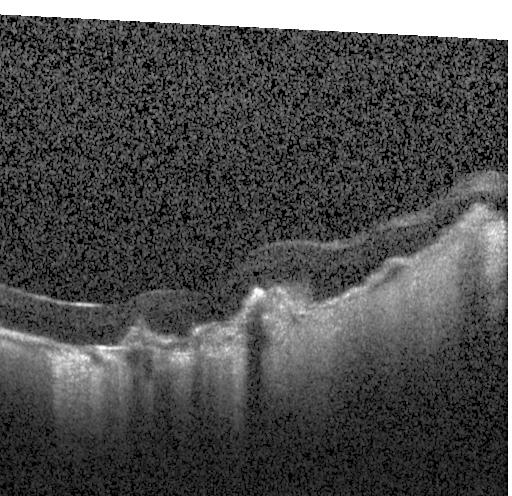
OCT finding: CNV.